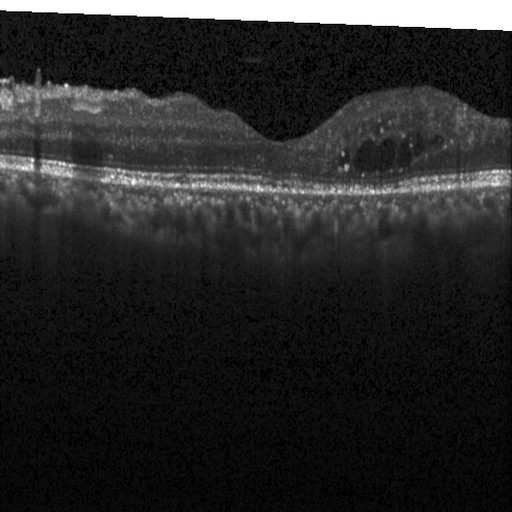
This B-scan demonstrates diabetic macular edema.